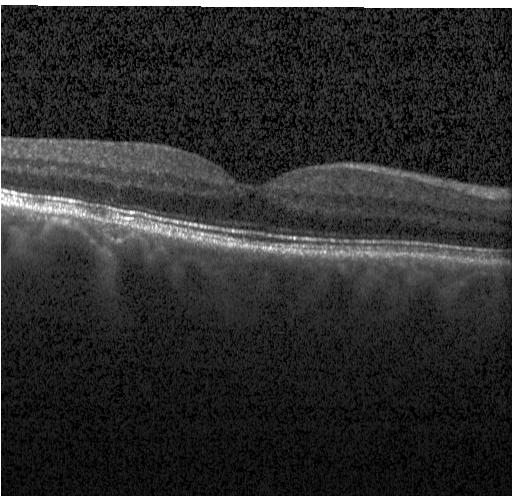
Macular OCT demonstrating no evidence of choroidal neovascularization, diabetic macular edema, or drusen.